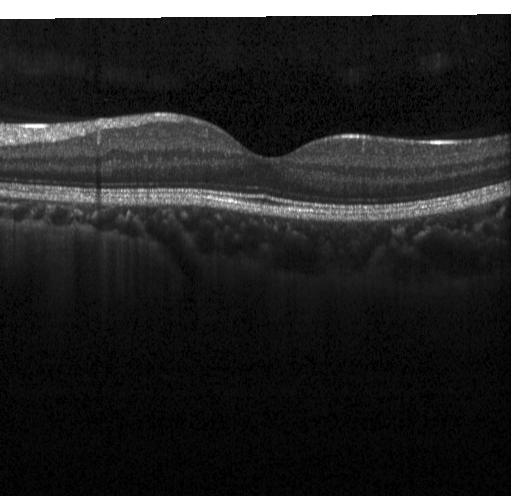
Optical coherence tomography B-scan.
Dx: neither choroidal neovascularization, diabetic macular edema, nor drusen.